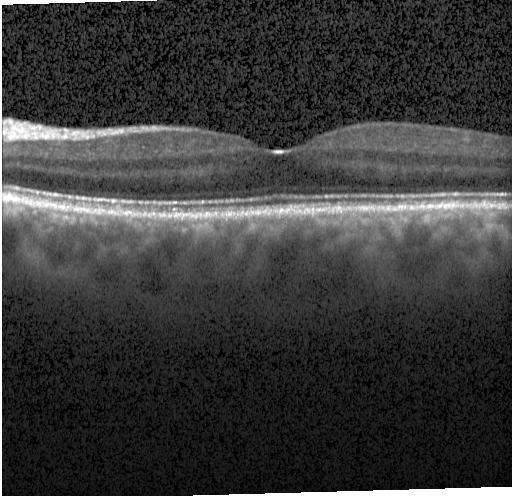

Spectral-domain OCT; acquired on a Heidelberg Spectralis; optical coherence tomography B-scan. The scan shows no choroidal neovascularization, diabetic macular edema, or drusen.